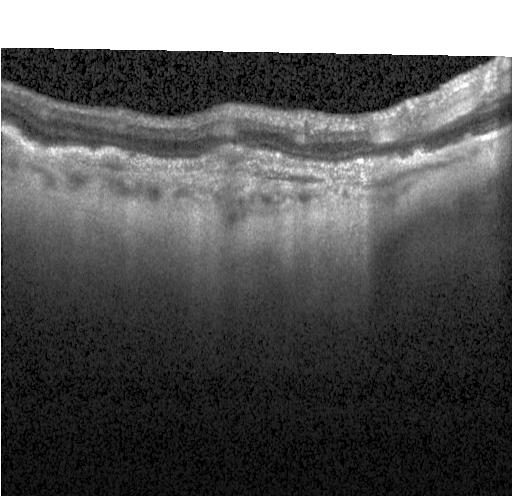
Spectral-domain OCT. Horizontal scan through the fovea. Retinal OCT B-scan. Instrument: Heidelberg Spectralis
Assessment: CNV.